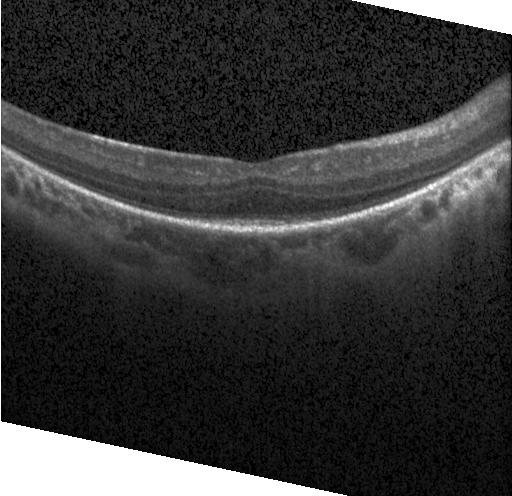 Through the macula, retinal OCT B-scan, spectral-domain optical coherence tomography — This B-scan demonstrates neither choroidal neovascularization, diabetic macular edema, nor drusen.